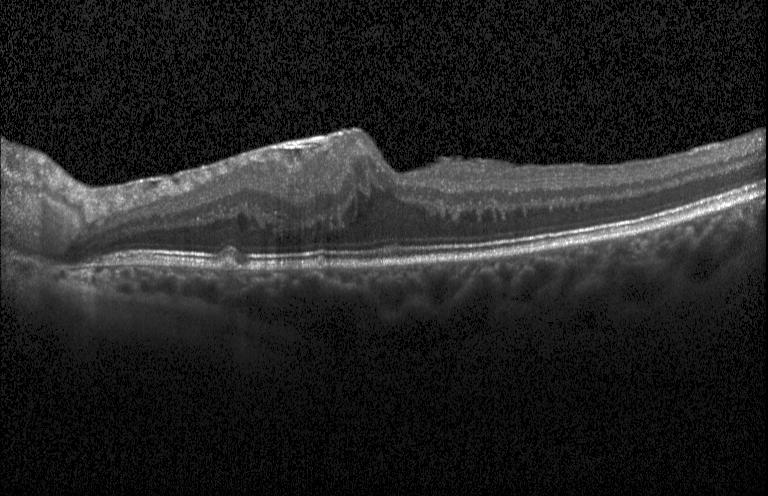

Diagnosis: multiple drusen.